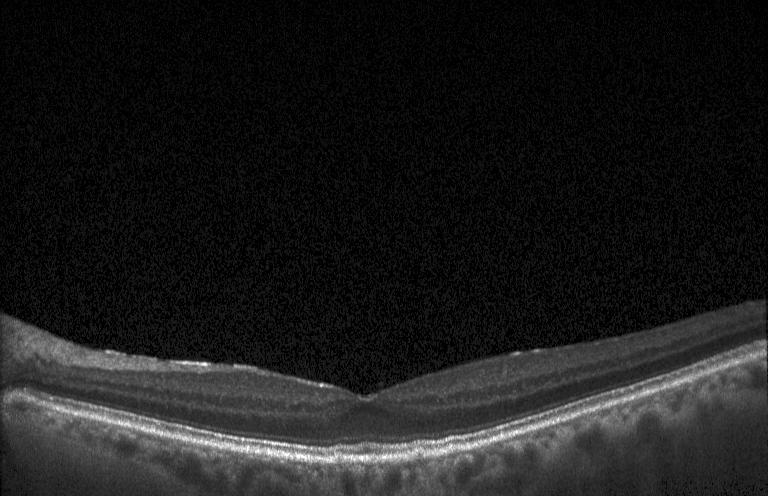

Retinal OCT cross-section, horizontal scan through the fovea, spectral-domain optical coherence tomography.
Finding: drusen.